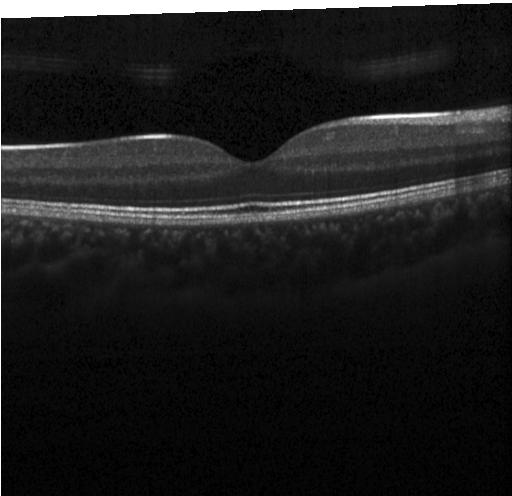

Retinal OCT B-scan. Finding: neither choroidal neovascularization, diabetic macular edema, nor drusen.